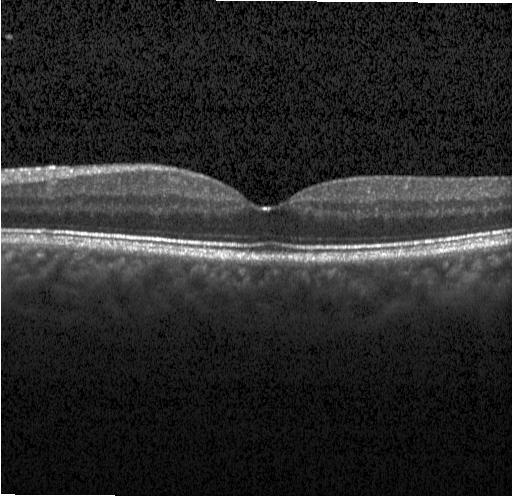

OCT scan showing no CNV, DME, or drusen.